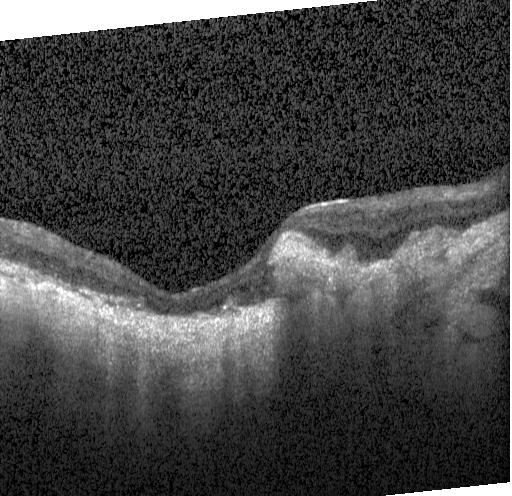
OCT finding: a choroidal neovascular membrane.